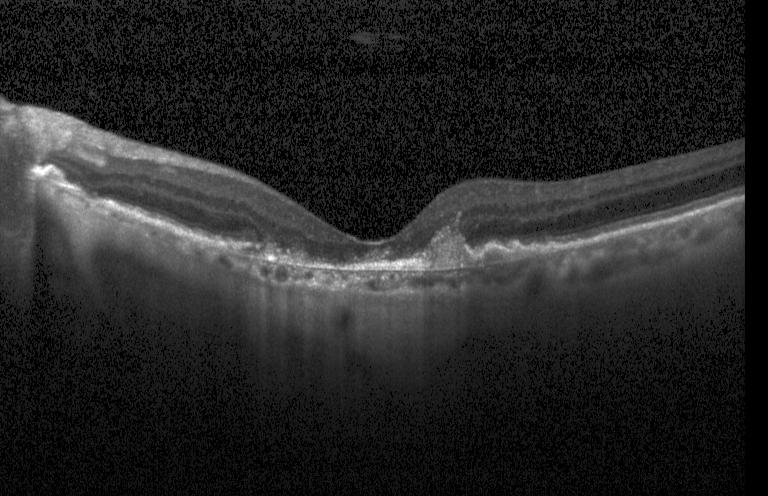
Heidelberg Spectralis · through the macula · SD-OCT · retinal OCT cross-section
The scan shows CNV.